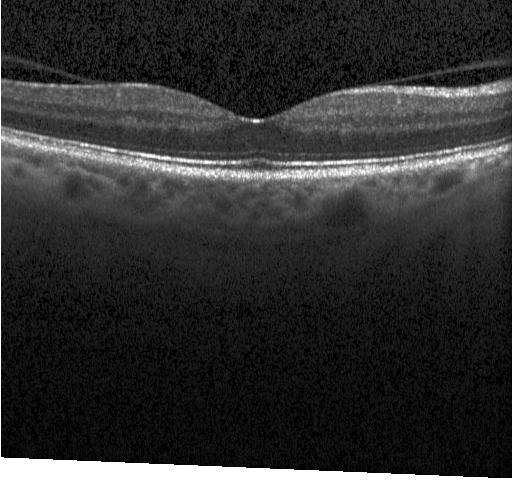

Finding: no choroidal neovascularization, diabetic macular edema, or drusen.